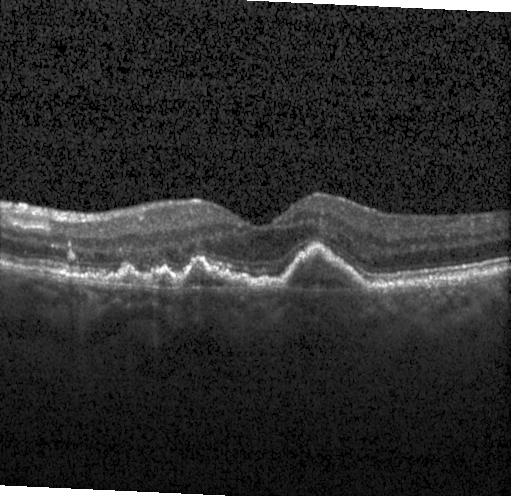 Horizontal scan through the fovea. Optical coherence tomography scan.
A choroidal neovascular membrane.